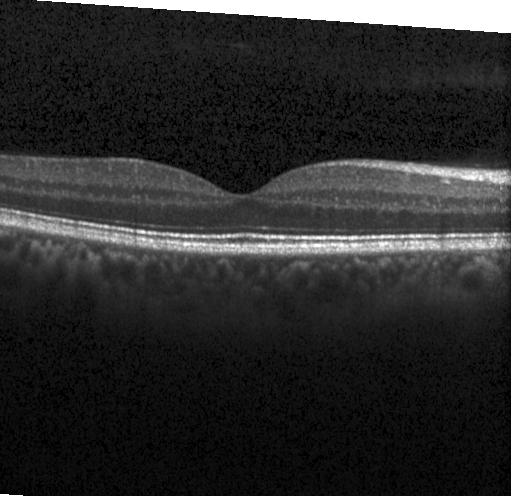
Heidelberg Spectralis OCT system · optical coherence tomography B-scan. No evidence of choroidal neovascularization, diabetic macular edema, or drusen.